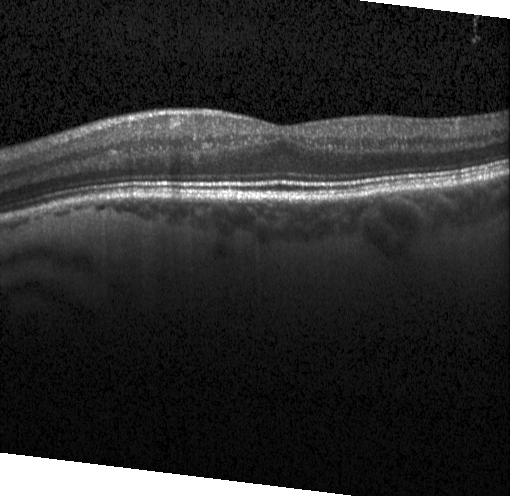 OCT finding: no evidence of CNV, DME, or drusen.